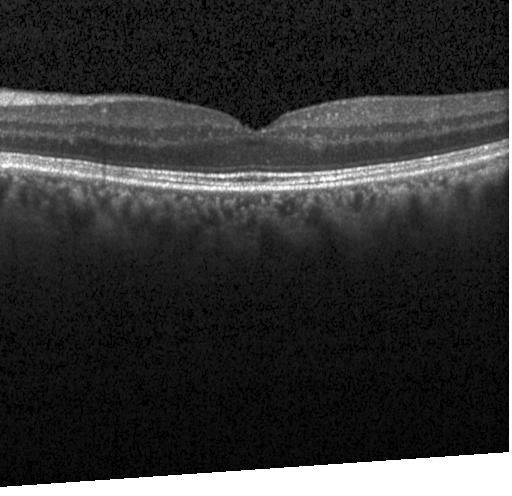

Impression: no evidence of choroidal neovascularization, diabetic macular edema, or drusen.